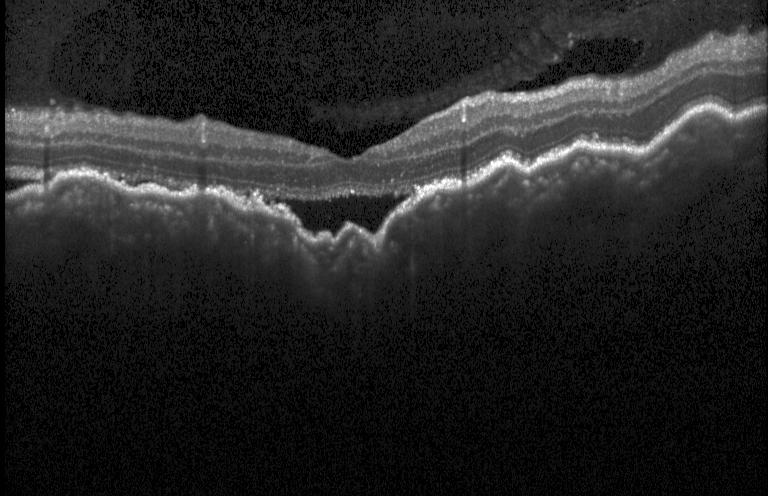
Centered on the fovea. Acquired on a Heidelberg Spectralis. OCT line scan. Spectral-domain OCT. This B-scan demonstrates choroidal neovascularization.